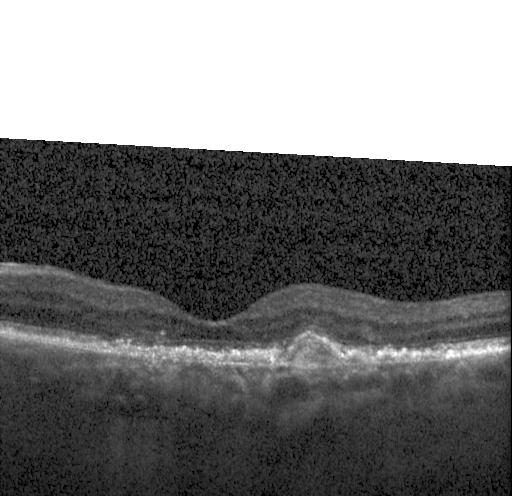 This B-scan demonstrates a choroidal neovascular membrane.